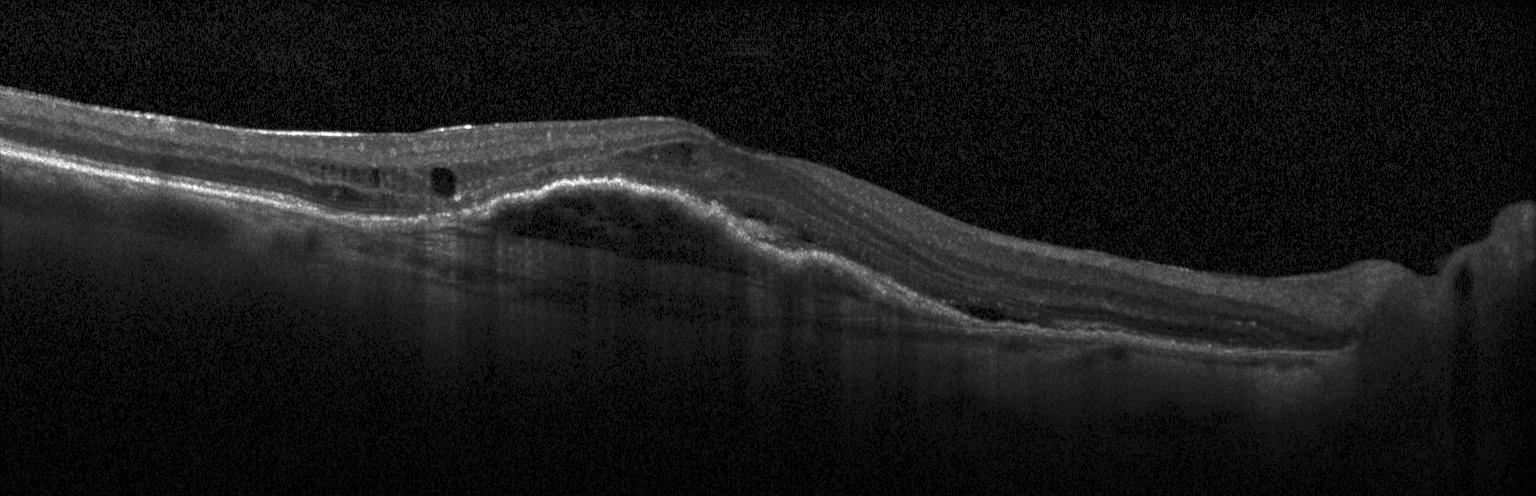 Retinal OCT B-scan. Instrument: Heidelberg Spectralis. Fovea-centered. SD-OCT — OCT finding: a choroidal neovascular membrane.